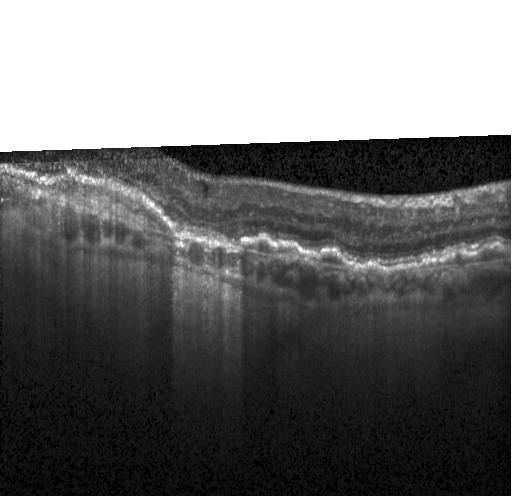
OCT B-scan.
Impression: a choroidal neovascular membrane.